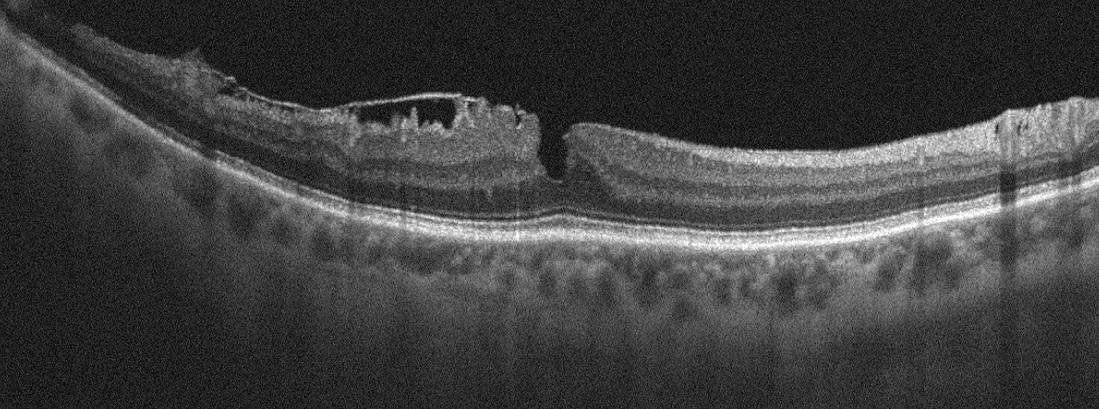 OCT B-scan · Optovue Avanti RTVue XR · fovea-centered. Finding: epiretinal membrane.